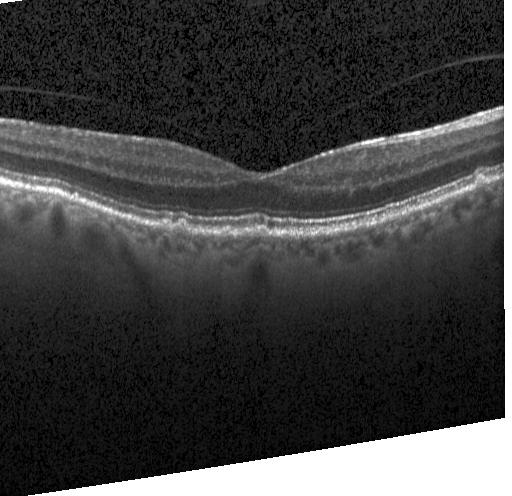 Spectral-domain OCT B-scan: drusen.